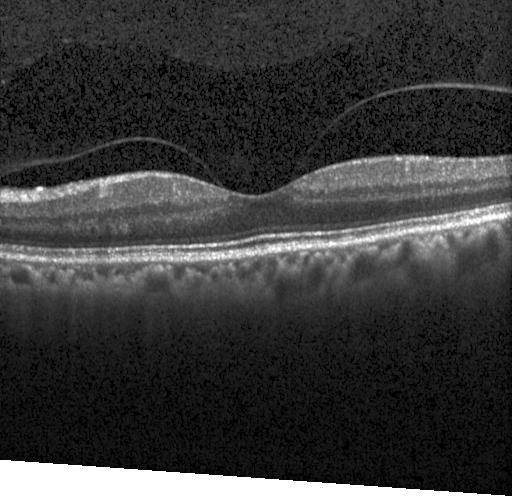

Diagnosis: no evidence of choroidal neovascularization, diabetic macular edema, or drusen.